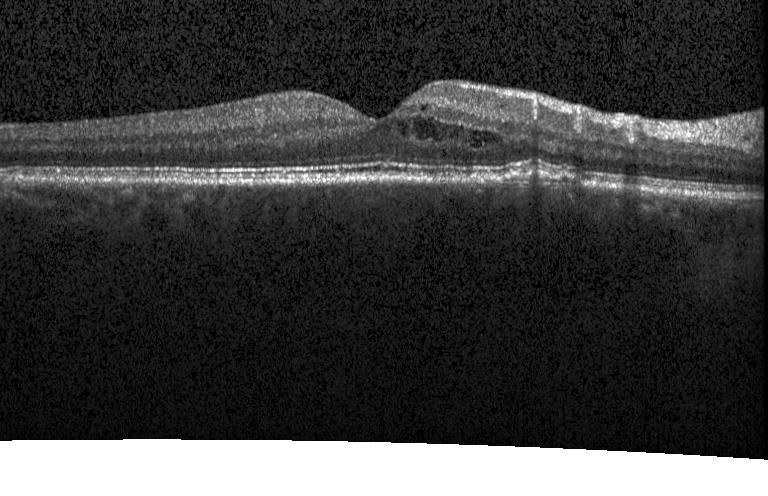

Retinal OCT B-scan.
Finding: a choroidal neovascular membrane.